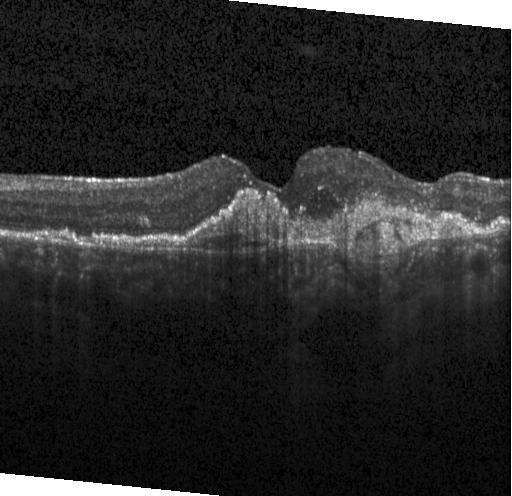
Impression: CNV.